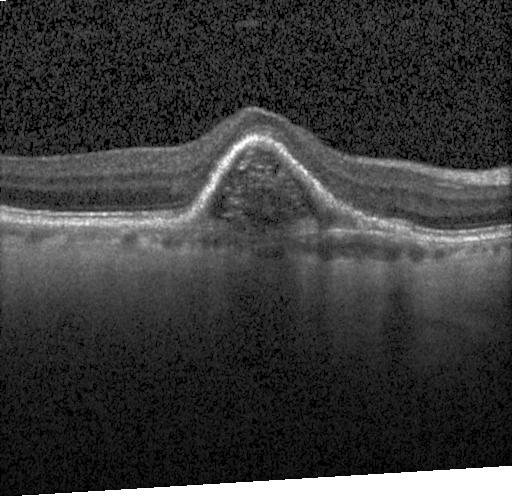
Optical coherence tomography scan, Heidelberg Spectralis OCT system, centered on the fovea — Diagnosis: a choroidal neovascular membrane.